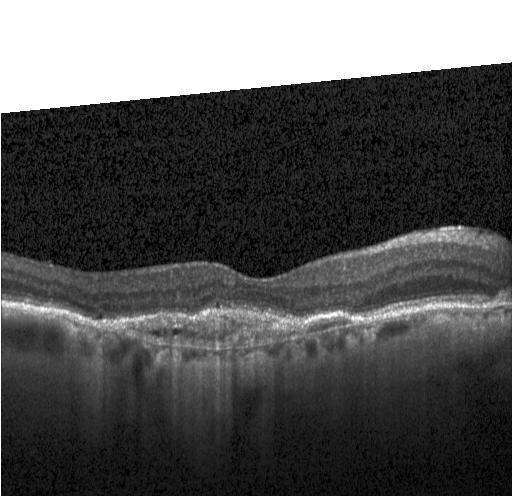 SD-OCT; horizontal scan through the fovea; OCT line scan — Diagnosis: a choroidal neovascular membrane.